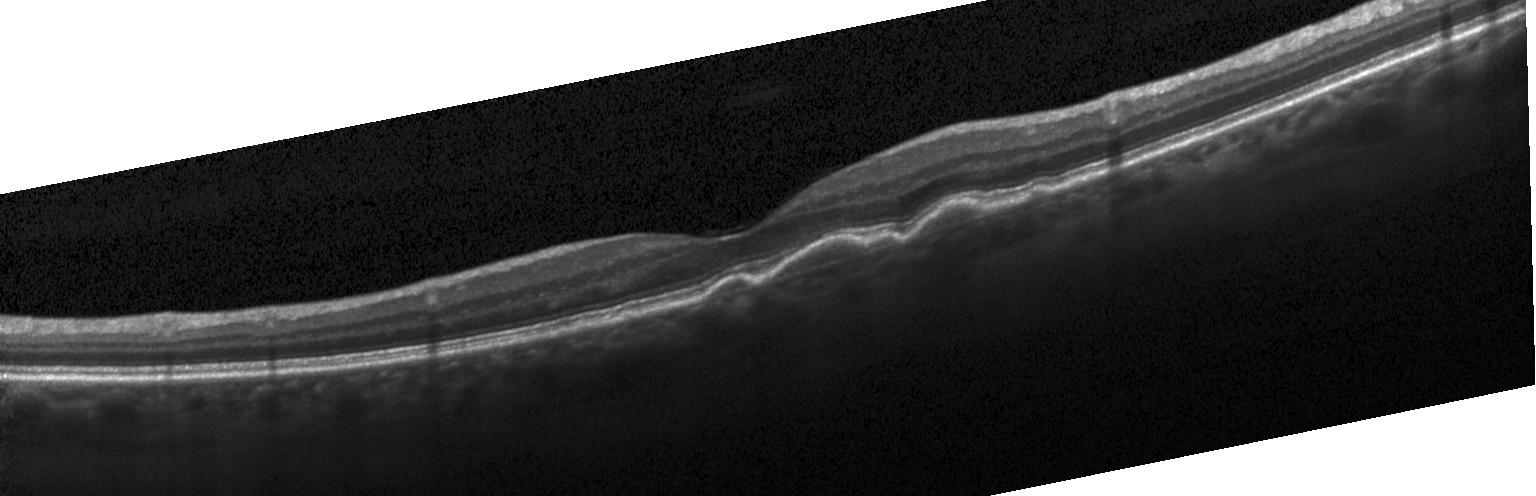
Fovea-centered · spectral-domain OCT · instrument: Heidelberg Spectralis · optical coherence tomography scan — This B-scan demonstrates a choroidal neovascular membrane.